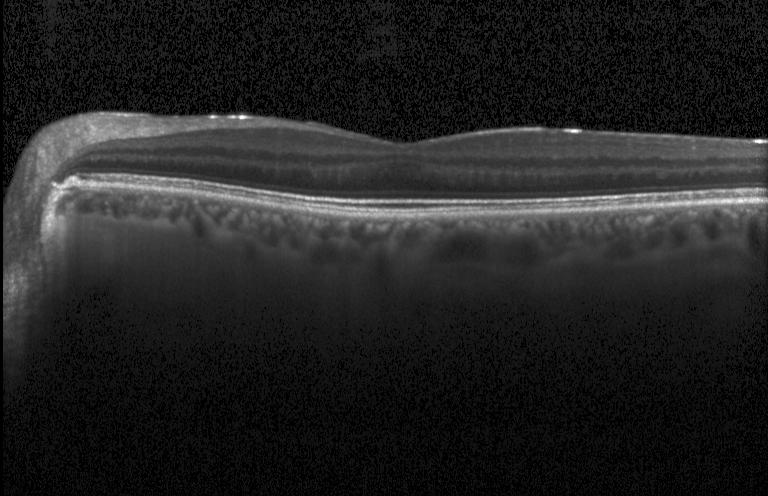 Spectral-domain OCT · OCT B-scan · acquired on a Heidelberg Spectralis. Diagnosis: no CNV, DME, or drusen.